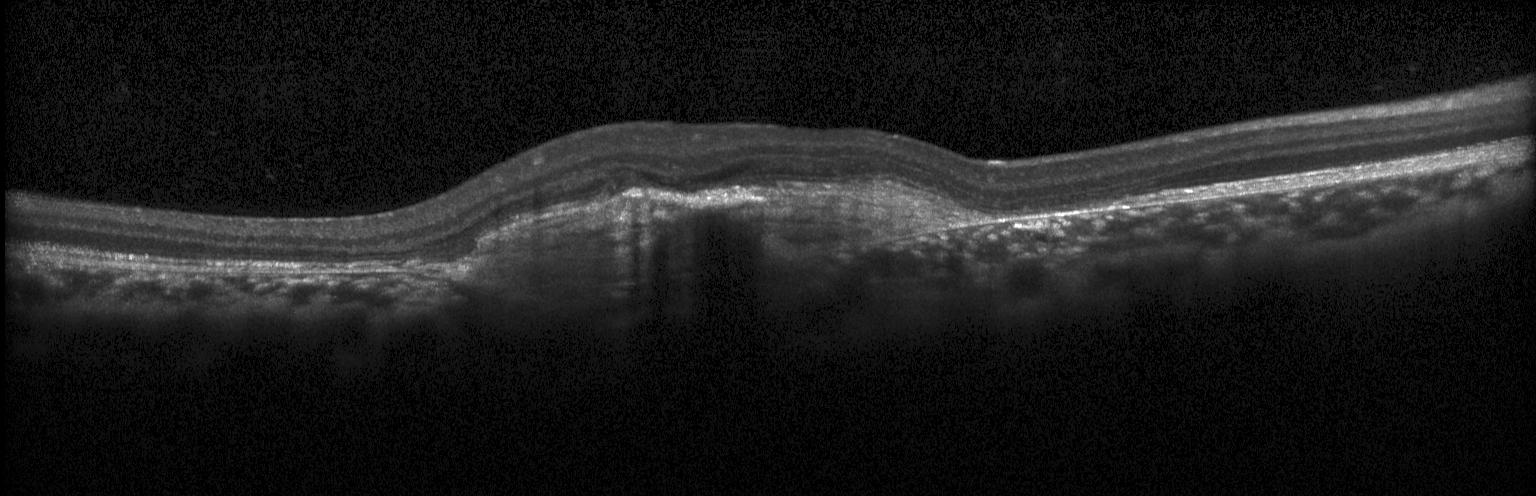

Fovea-centered, OCT B-scan, spectral-domain optical coherence tomography
OCT finding: a choroidal neovascular membrane.